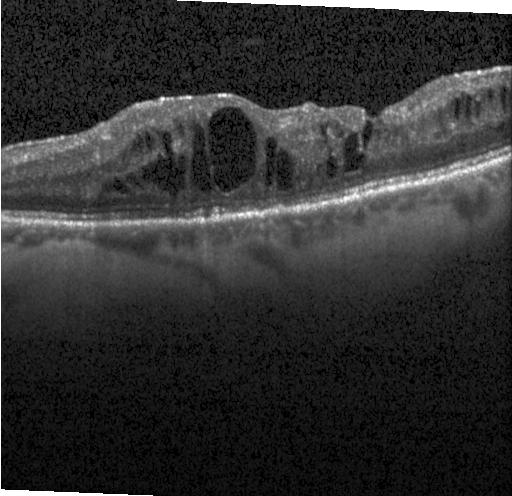

Through the macula · OCT line scan · spectral-domain OCT — DME.